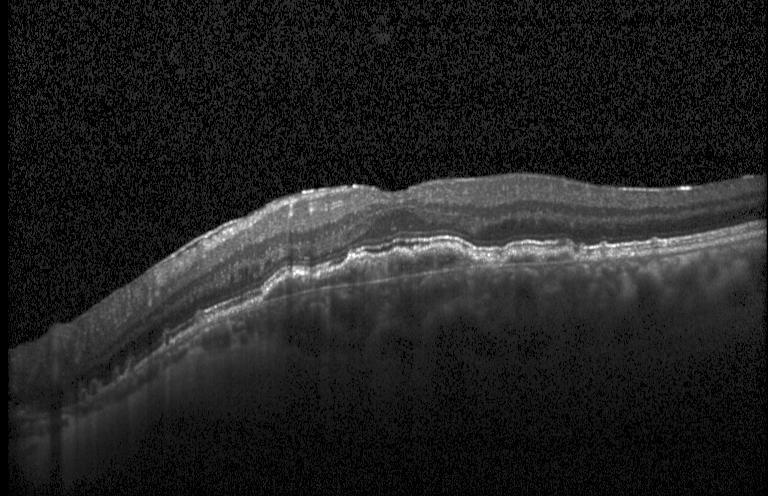

Diagnosis: choroidal neovascularization.